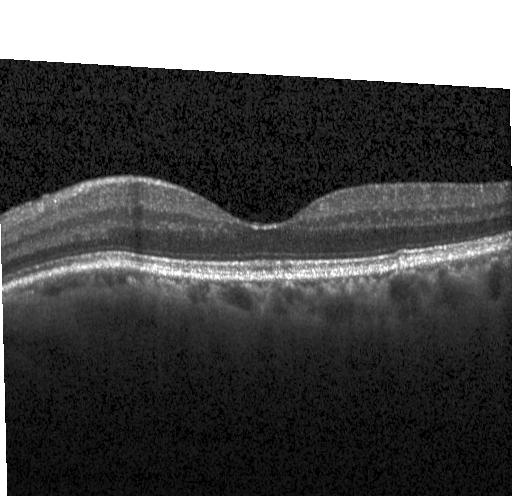 Retinal OCT cross-section showing no evidence of choroidal neovascularization, diabetic macular edema, or drusen.